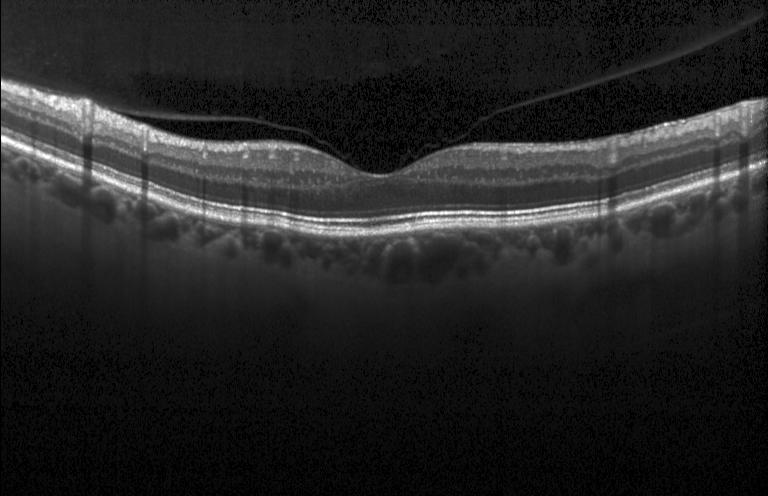
OCT line scan — Finding: no choroidal neovascularization, no diabetic macular edema, and no drusen.